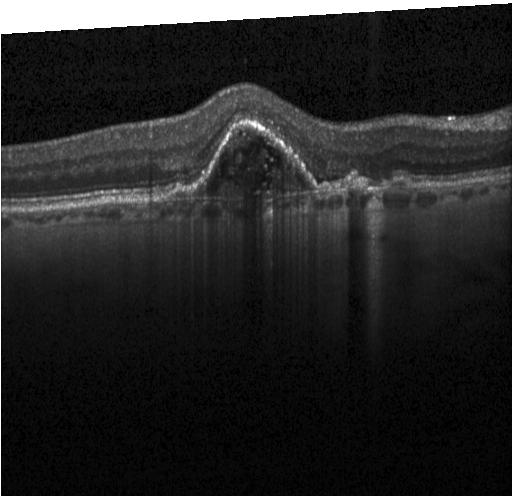

OCT finding: a choroidal neovascular membrane.